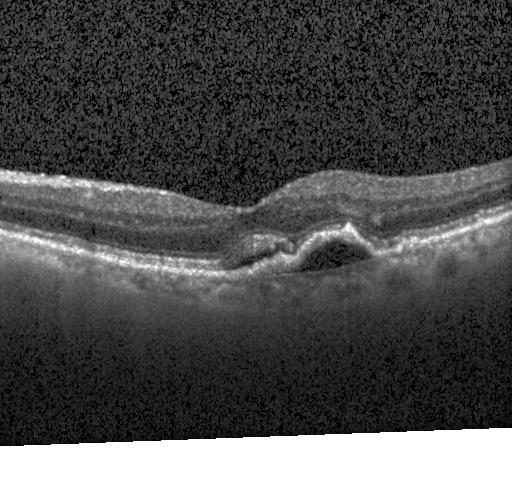 Spectral-domain OCT; retinal OCT B-scan. Assessment: choroidal neovascularization (CNV).